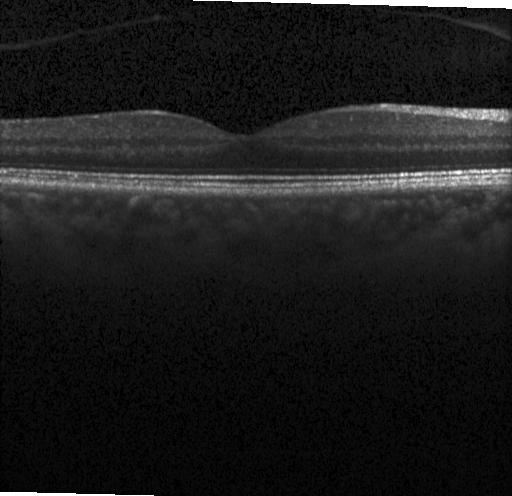 OCT B-scan. Heidelberg Spectralis. Spectral-domain optical coherence tomography. Fovea-centered. OCT finding: no choroidal neovascularization, no diabetic macular edema, and no drusen.